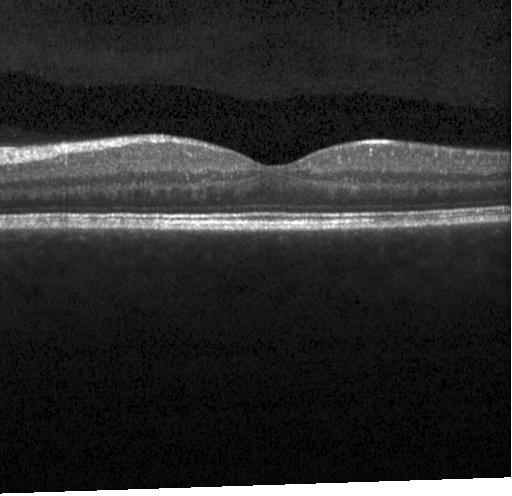

Retinal OCT B-scan
Finding: neither choroidal neovascularization, diabetic macular edema, nor drusen.